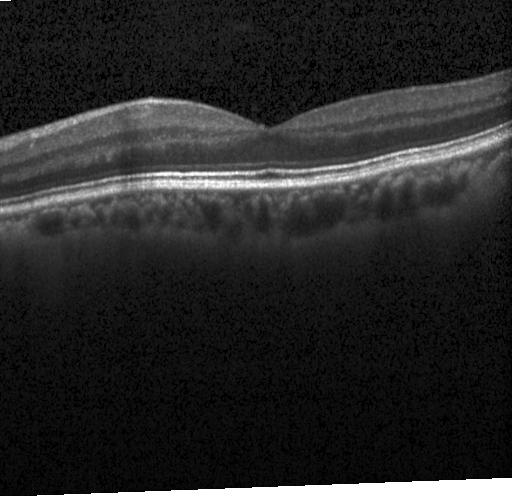
Acquired on a Heidelberg Spectralis · retinal OCT cross-section · SD-OCT — Neither CNV, DME, nor drusen.